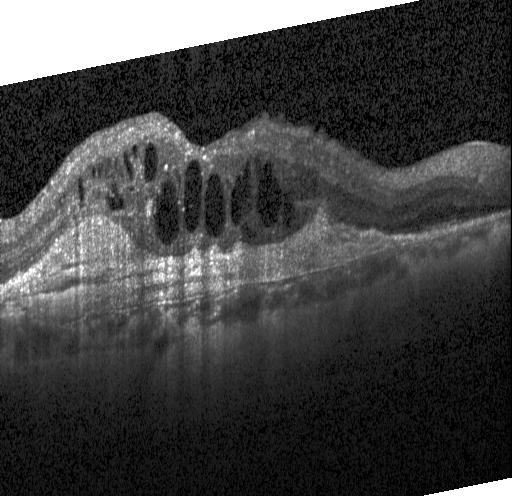
Dx: a choroidal neovascular membrane.